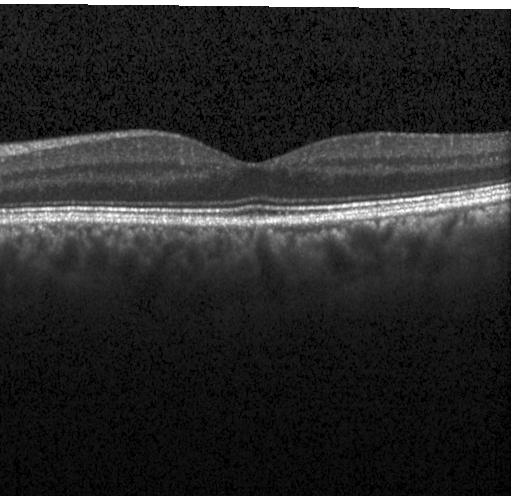
Retinal OCT cross-section showing no evidence of choroidal neovascularization, diabetic macular edema, or drusen.